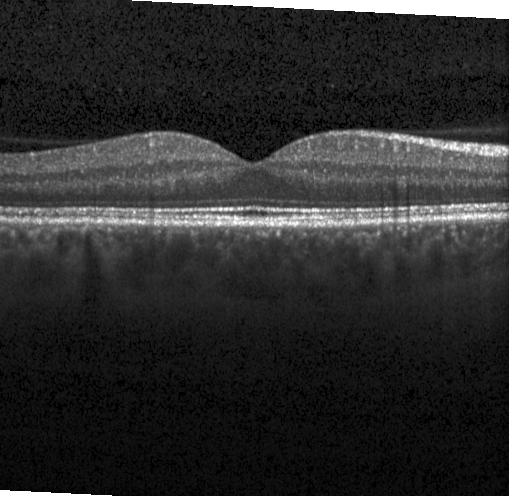

Finding: no choroidal neovascularization, diabetic macular edema, or drusen.